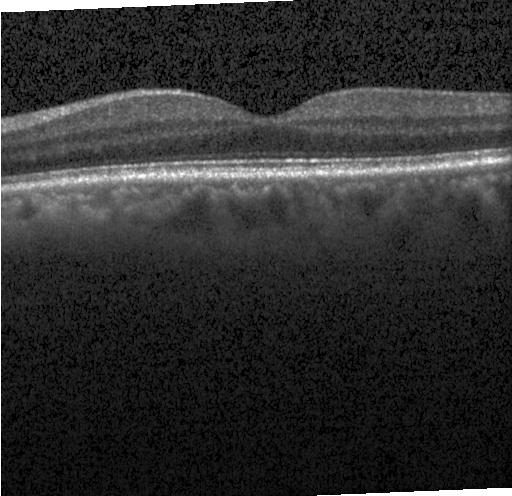

Spectral-domain optical coherence tomography. Instrument: Heidelberg Spectralis. Retinal OCT B-scan.
Impression: no CNV, DME, or drusen.